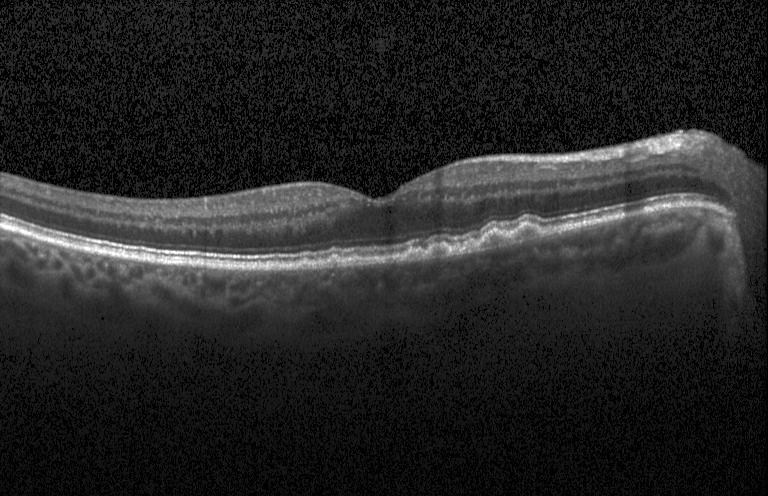

Acquired on a Heidelberg Spectralis; horizontal scan through the fovea; OCT line scan; spectral-domain optical coherence tomography — Impression: drusen.